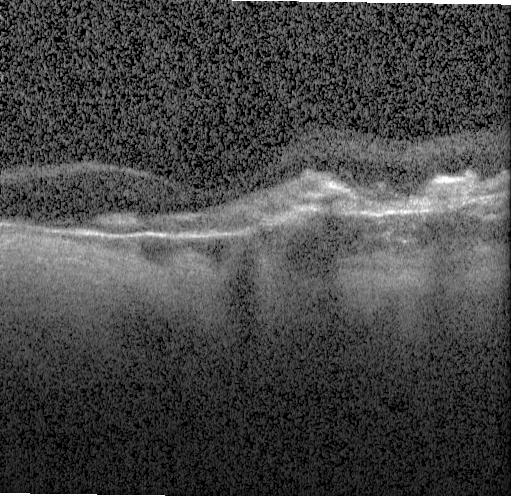 Through the macula, OCT B-scan, Heidelberg Spectralis OCT system, spectral-domain optical coherence tomography.
Diagnosis: a choroidal neovascular membrane.